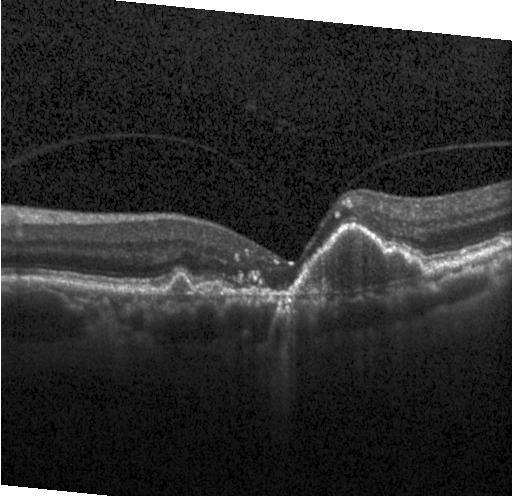 Macular OCT: a choroidal neovascular membrane.